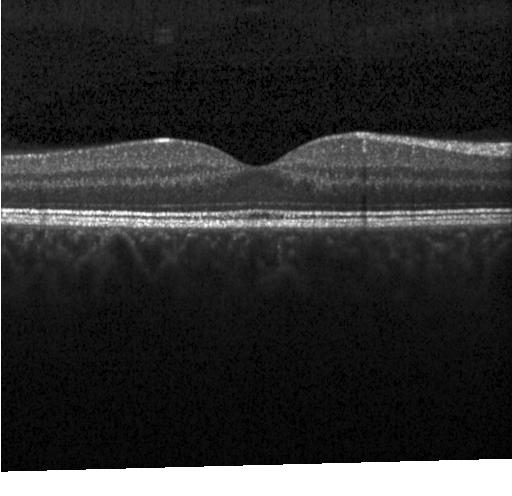
Instrument: Heidelberg Spectralis. Spectral-domain OCT. Through the macula. Retinal OCT cross-section
Finding: no evidence of choroidal neovascularization, diabetic macular edema, or drusen.